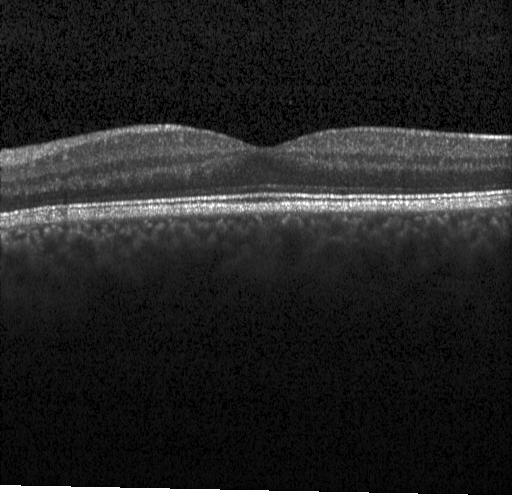

OCT line scan. SD-OCT. Impression: no evidence of choroidal neovascularization, diabetic macular edema, or drusen.